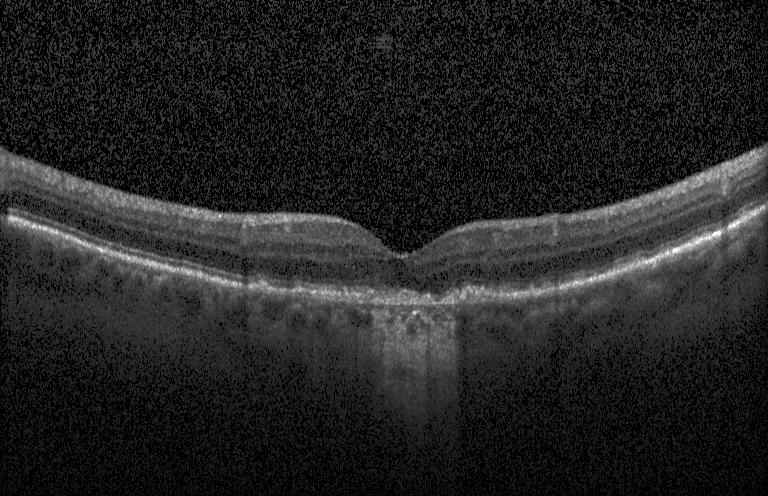

Horizontal scan through the fovea, optical coherence tomography scan, spectral-domain optical coherence tomography. The scan shows choroidal neovascularization (CNV).